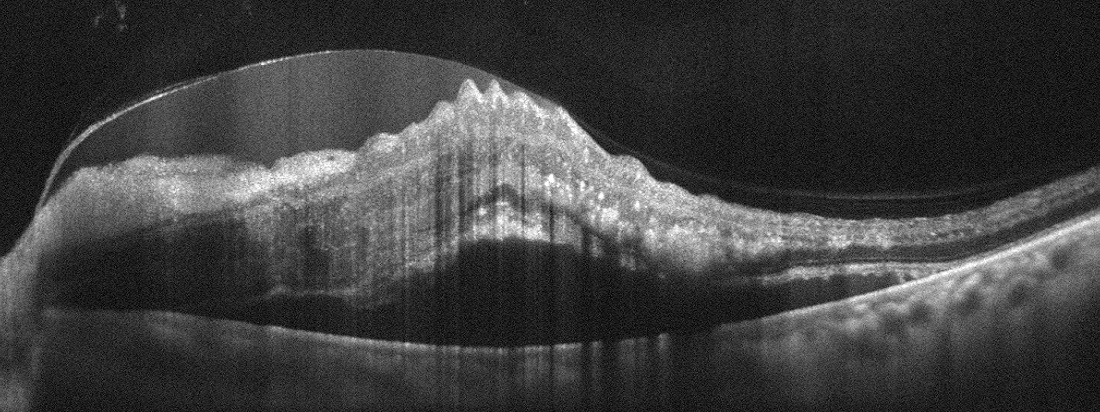
OCT line scan. Through the macula. Impression: RVO.